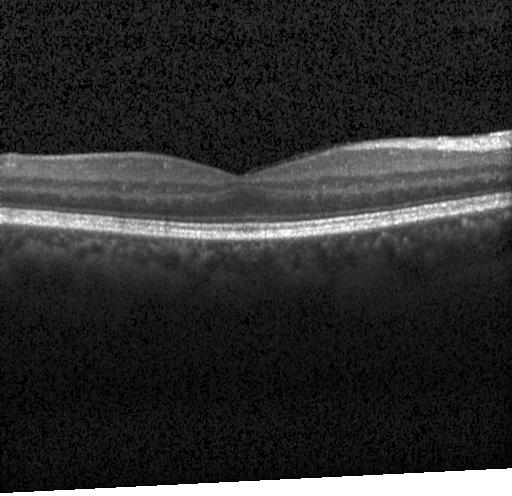
Impression: neither CNV, DME, nor drusen.